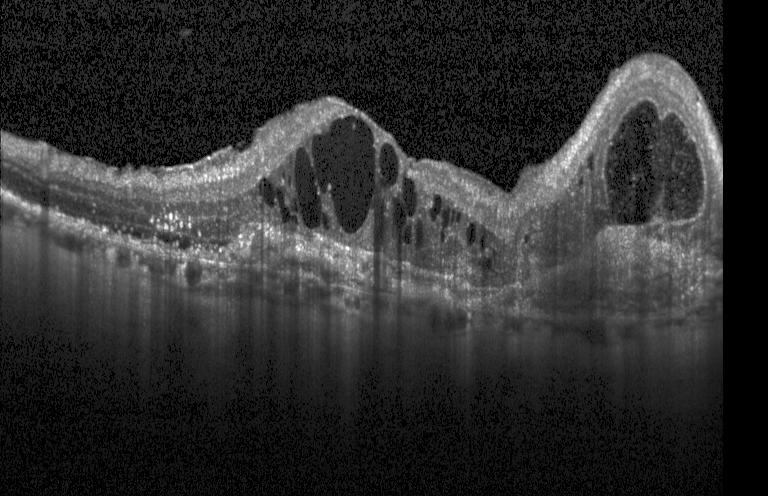

Spectral-domain optical coherence tomography; OCT B-scan. This B-scan demonstrates choroidal neovascularization (CNV).